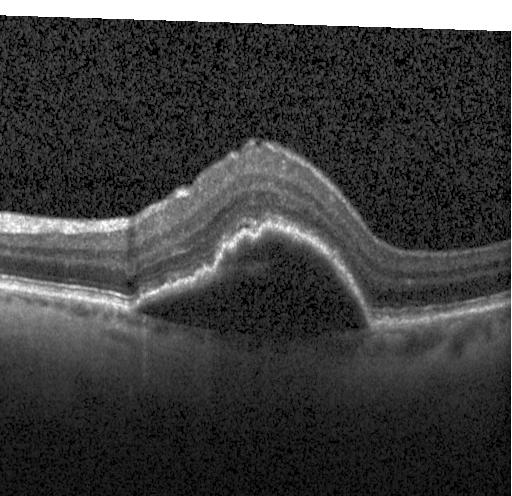 Assessment: choroidal neovascularization.